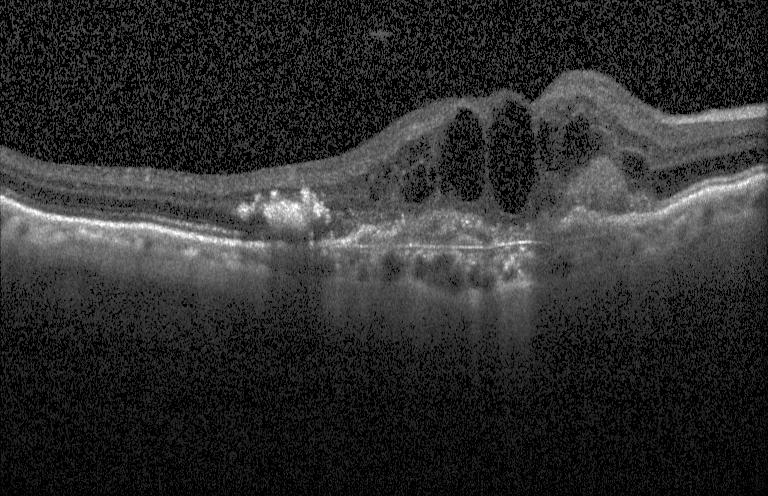

SD-OCT. Optical coherence tomography B-scan. Acquired on a Heidelberg Spectralis — Impression: CNV.